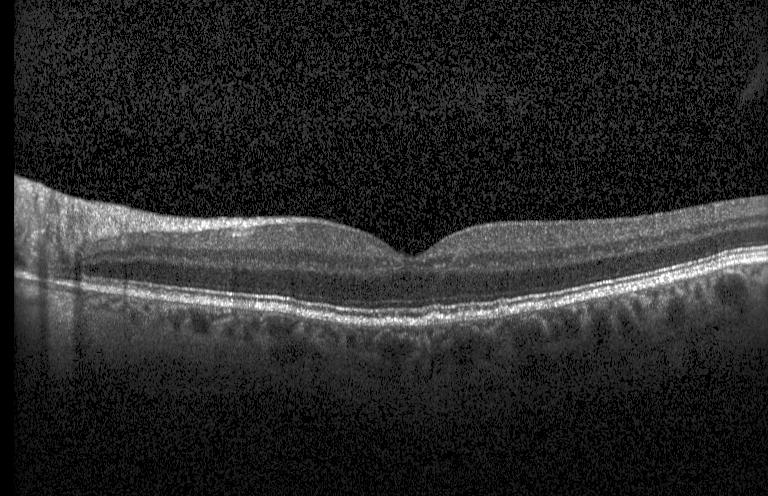
Instrument: Heidelberg Spectralis, optical coherence tomography B-scan, SD-OCT, fovea-centered. Impression: multiple drusen.